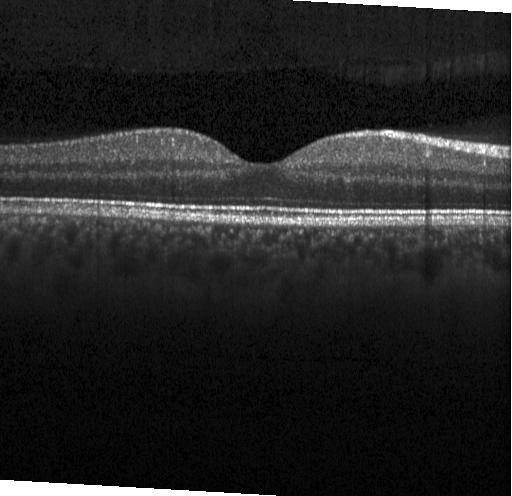
Spectral-domain optical coherence tomography. Instrument: Heidelberg Spectralis. Optical coherence tomography B-scan.
Neither choroidal neovascularization, diabetic macular edema, nor drusen.